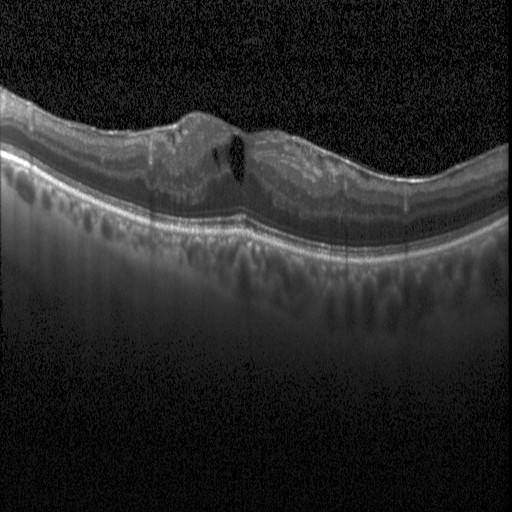
Instrument: Heidelberg Spectralis · optical coherence tomography scan · spectral-domain optical coherence tomography · centered on the fovea — Diagnosis: diabetic macular edema (DME).